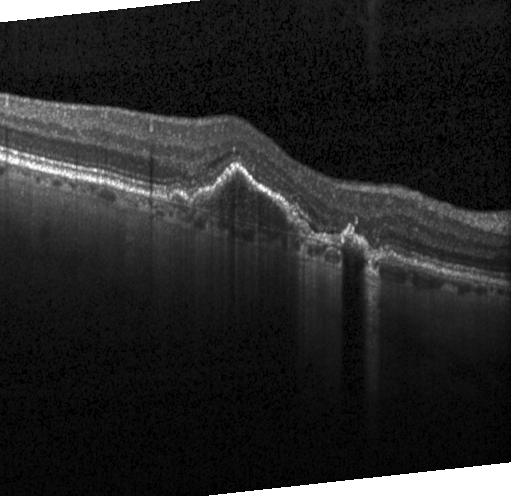 Optical coherence tomography B-scan. Impression: a choroidal neovascular membrane.